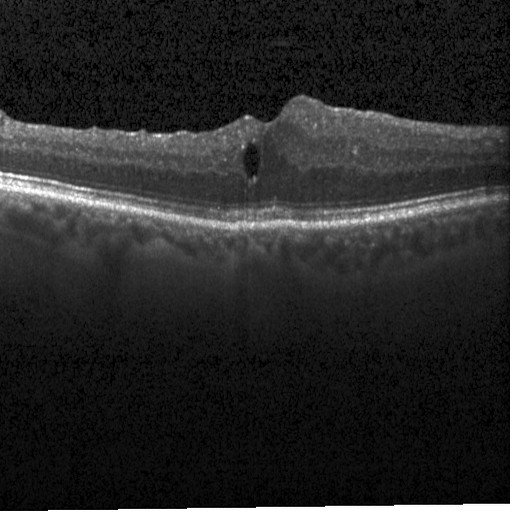 Optical coherence tomography scan. Instrument: Heidelberg Spectralis
Macular OCT: diabetic macular edema.